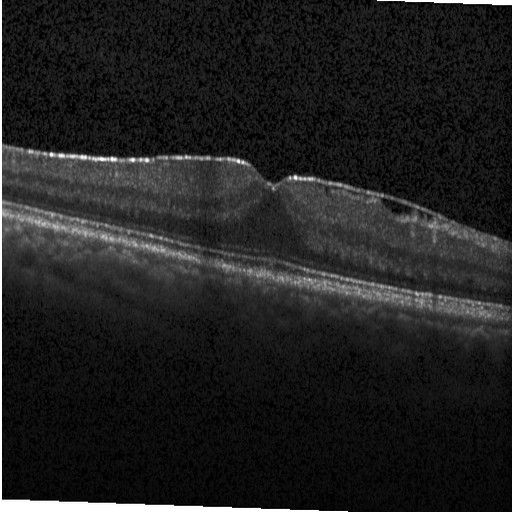

Retinal OCT cross-section. Diagnosis: diabetic macular edema.